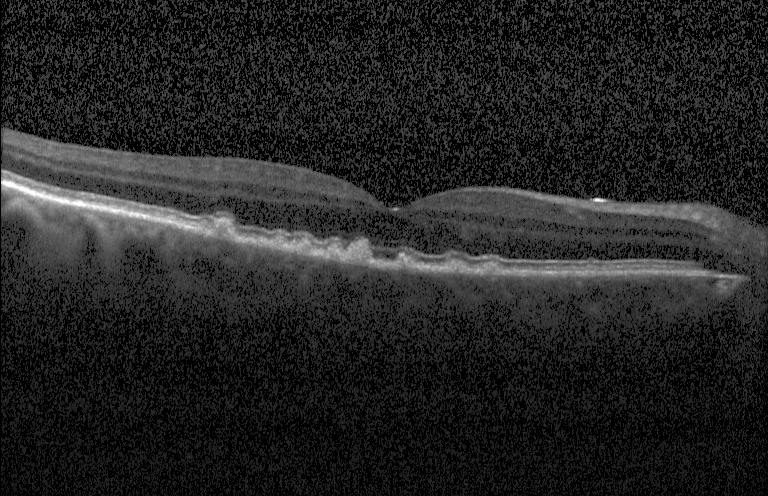 Retinal OCT cross-section · Heidelberg Spectralis · spectral-domain optical coherence tomography · through the macula — OCT finding: sub-RPE drusenoid deposits.